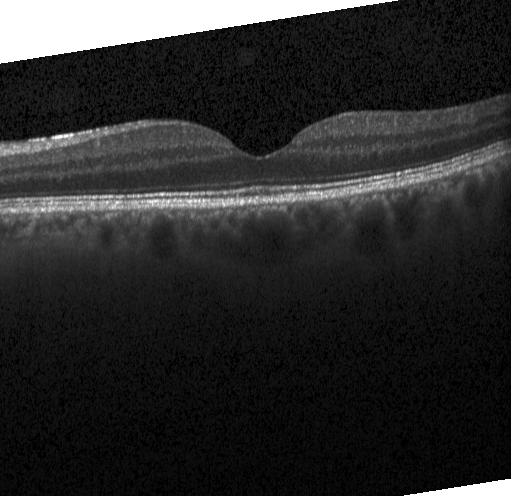
No evidence of choroidal neovascularization, diabetic macular edema, or drusen.